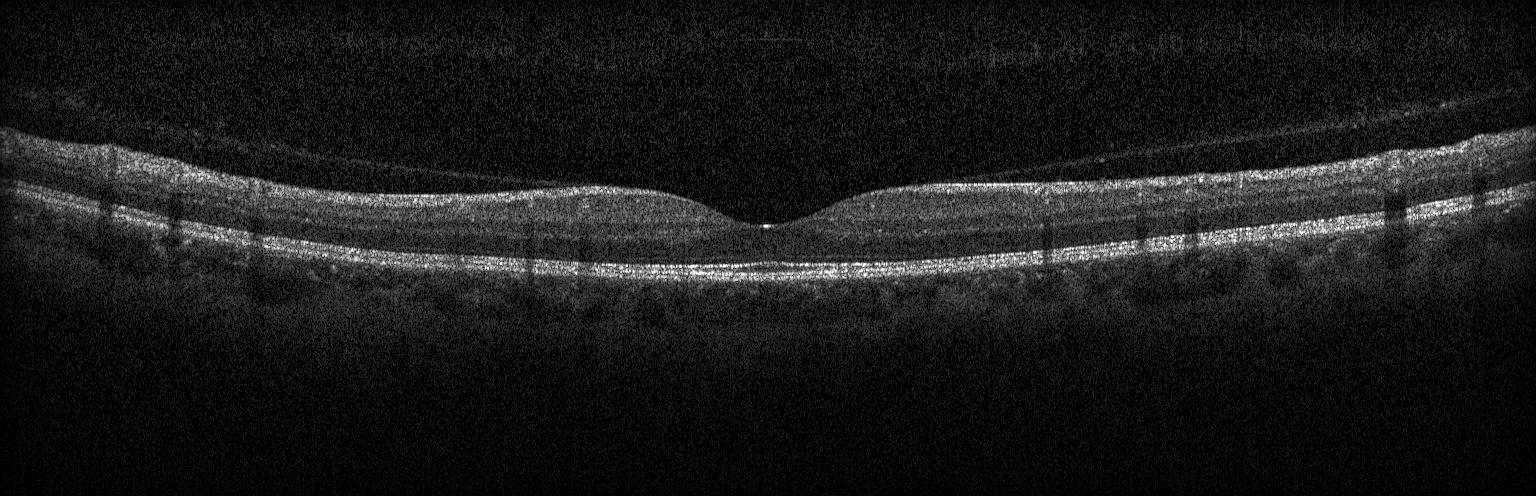 Spectral-domain OCT, retinal OCT B-scan, through the macula
Impression: no CNV, no DME, and no drusen.